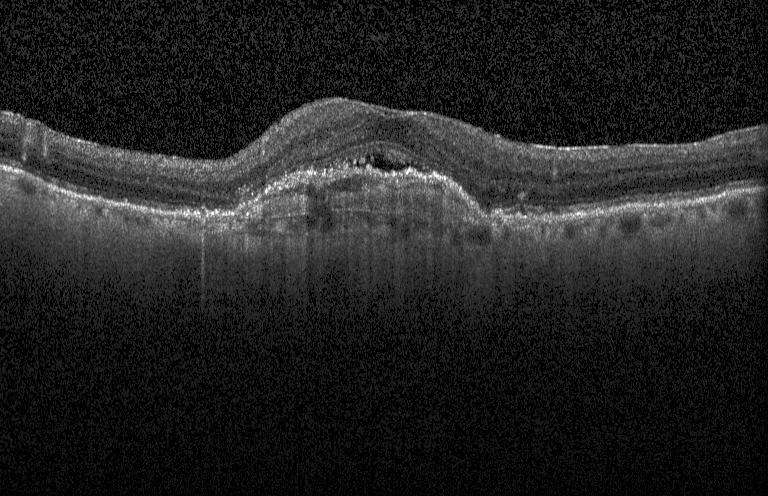
This B-scan demonstrates choroidal neovascularization.